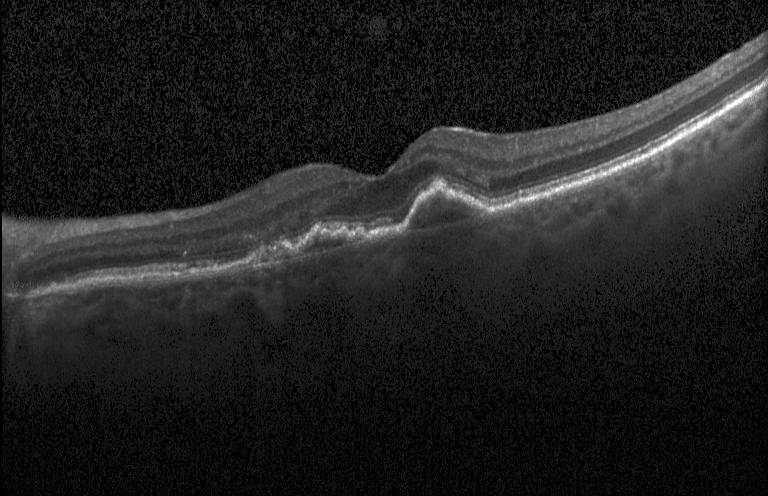 Retinal OCT cross-section. Through the macula
Impression: a choroidal neovascular membrane.